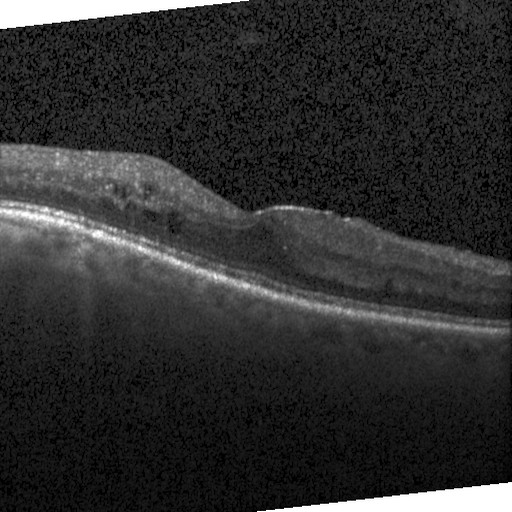 Through the macula; optical coherence tomography scan.
This B-scan demonstrates DME.